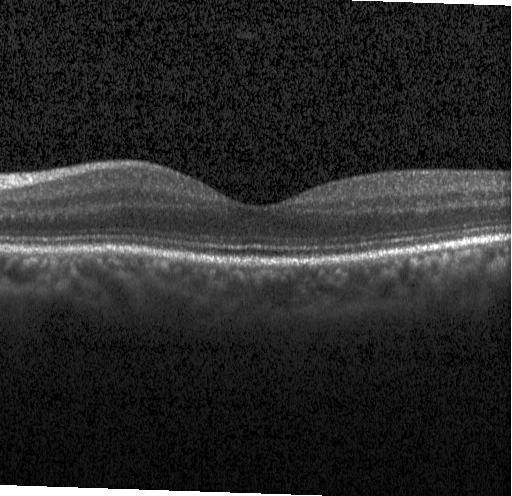

Retinal OCT B-scan, spectral-domain optical coherence tomography — Finding: no choroidal neovascularization, diabetic macular edema, or drusen.